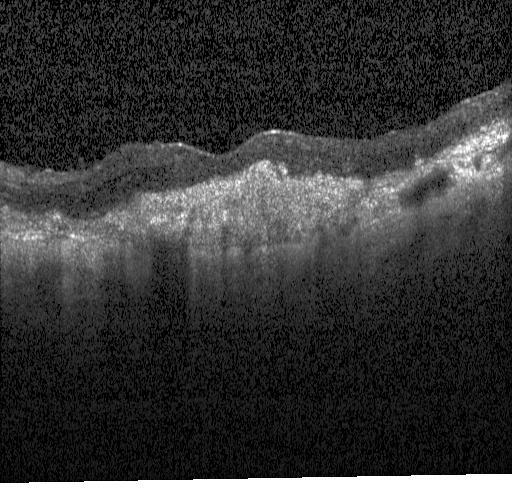
This B-scan demonstrates CNV.